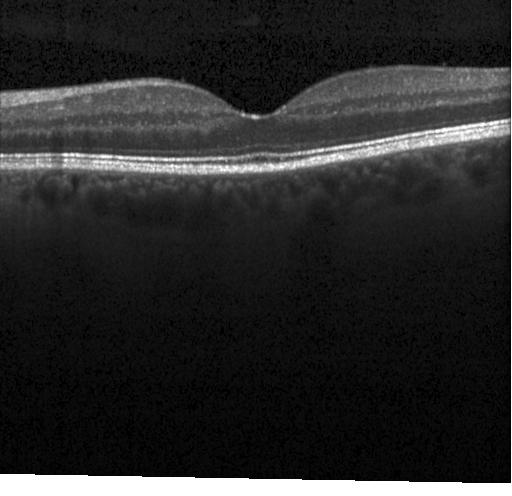 No evidence of choroidal neovascularization, diabetic macular edema, or drusen.